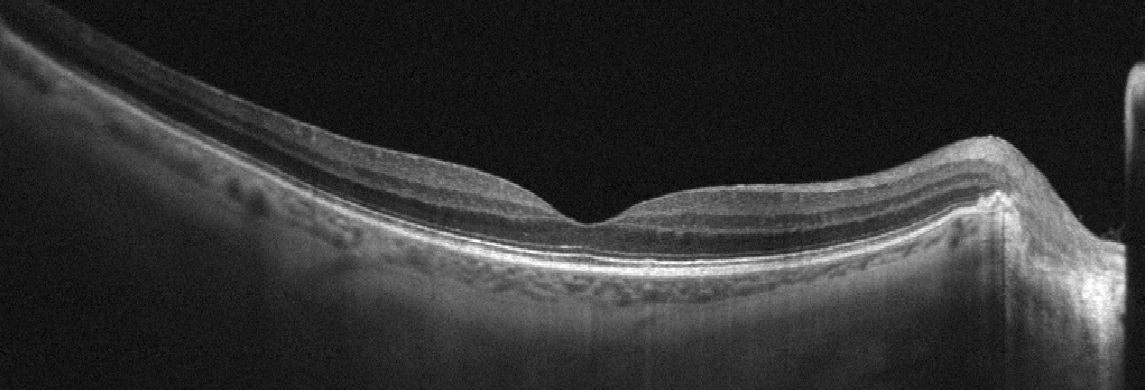
Impression: age-related macular degeneration.